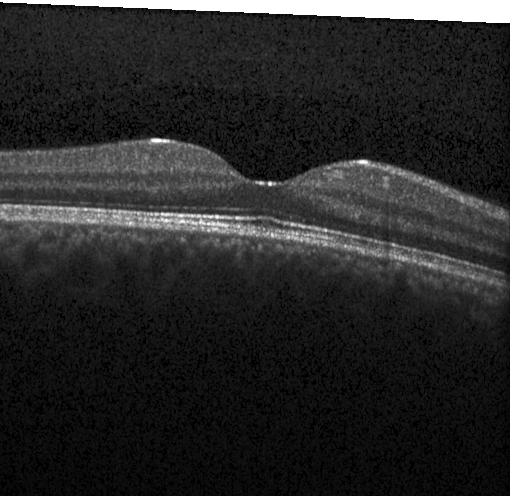 Retinal OCT cross-section.
OCT finding: no choroidal neovascularization, no diabetic macular edema, and no drusen.